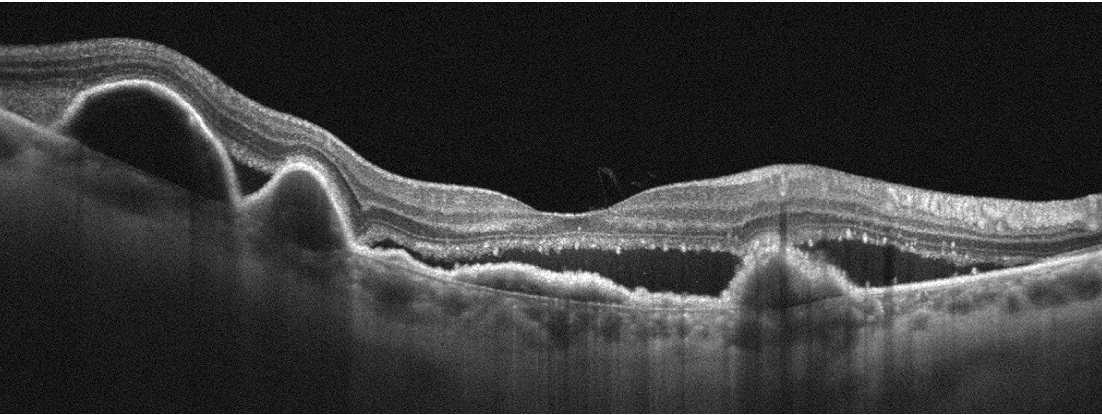
Retinal OCT cross-section
OCT finding: age-related macular degeneration.